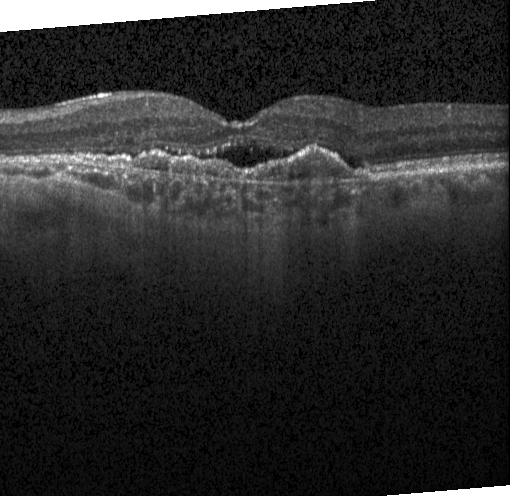 Optical coherence tomography B-scan. Instrument: Heidelberg Spectralis. Macular scan.
Diagnosis: choroidal neovascularization (CNV).